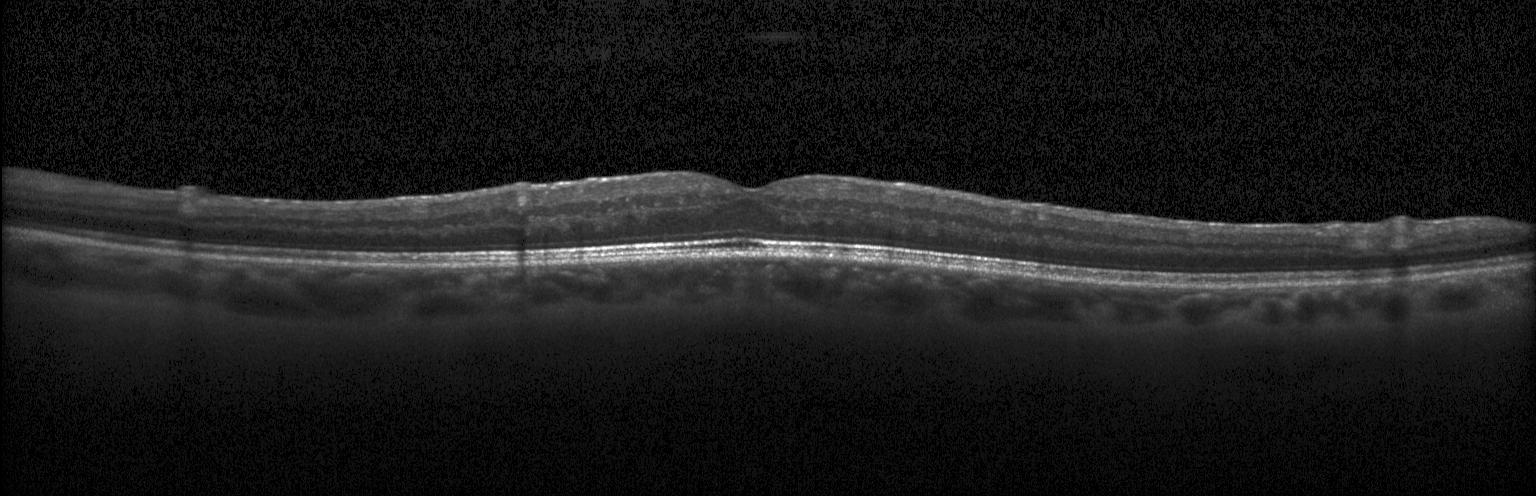

Diagnosis: no choroidal neovascularization, diabetic macular edema, or drusen.